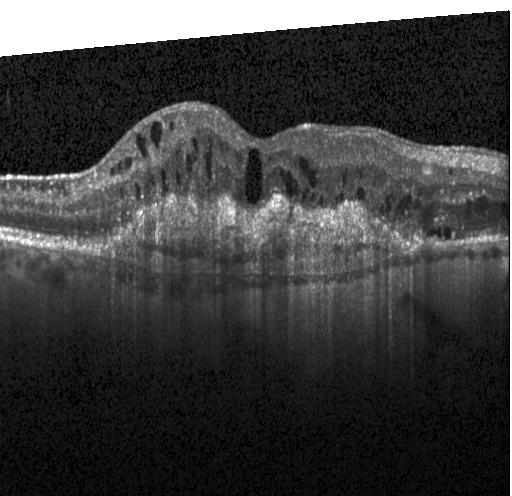 Heidelberg Spectralis, retinal OCT B-scan.
Impression: a choroidal neovascular membrane.